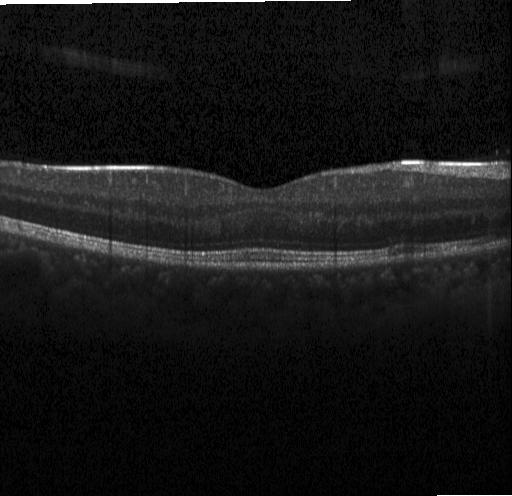
This B-scan demonstrates no CNV, DME, or drusen.